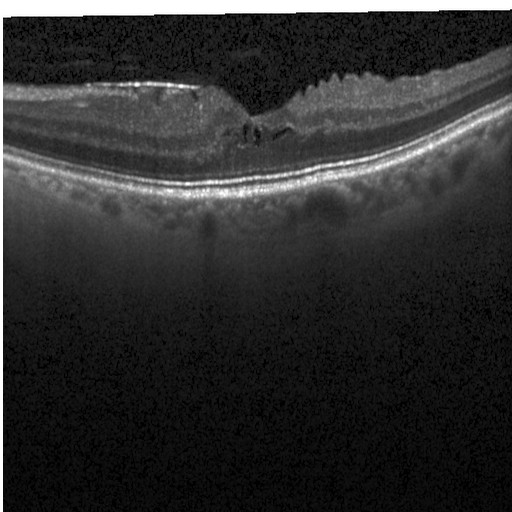
Retinal OCT cross-section showing diabetic macular edema.